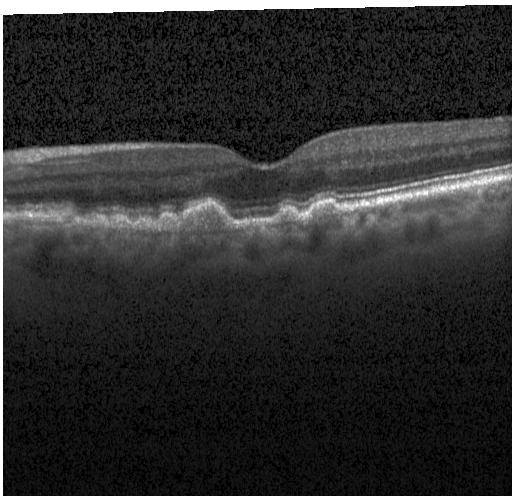 Heidelberg Spectralis; OCT B-scan.
Diagnosis: sub-RPE drusenoid deposits.